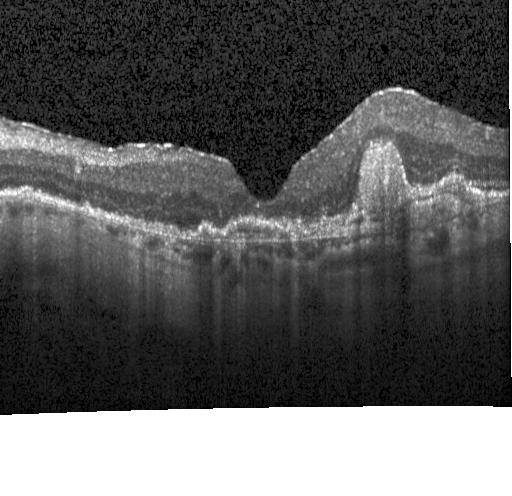 Assessment: CNV.